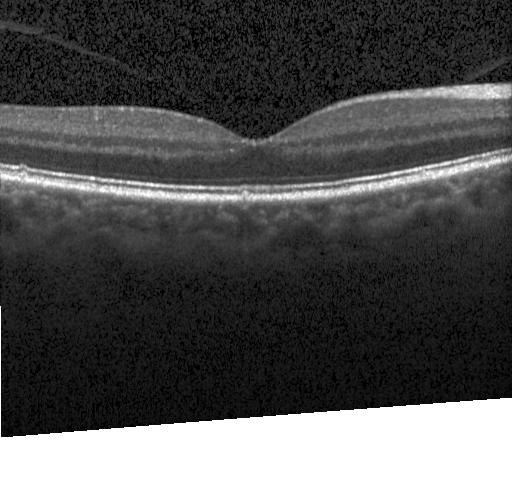

Spectral-domain OCT B-scan: multiple drusen.